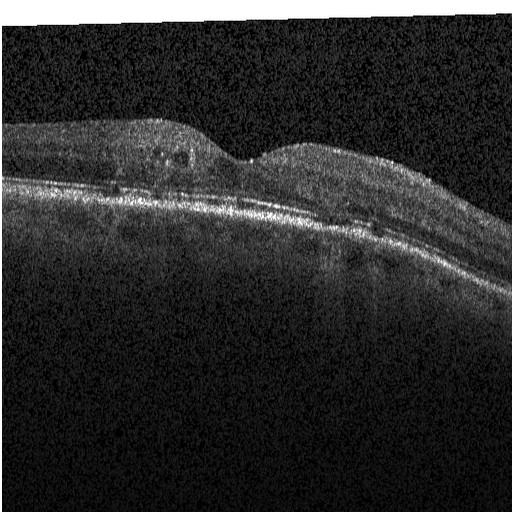

Through the macula, retinal OCT B-scan, spectral-domain OCT.
Finding: DME.